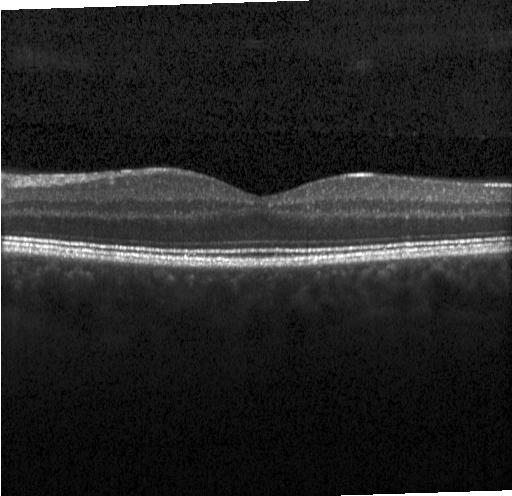
Optical coherence tomography B-scan; SD-OCT; fovea-centered; acquired on a Heidelberg Spectralis.
This B-scan demonstrates neither choroidal neovascularization, diabetic macular edema, nor drusen.